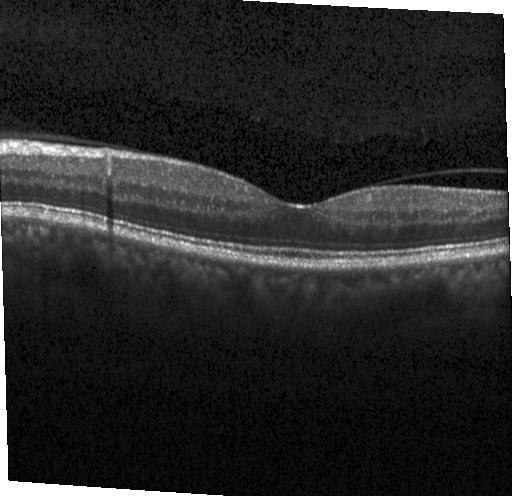 Impression: no CNV, no DME, and no drusen.